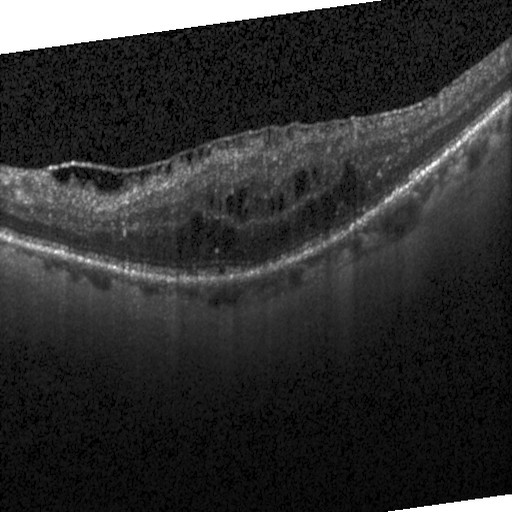

OCT B-scan, through the macula, Heidelberg Spectralis, SD-OCT
This B-scan demonstrates DME.